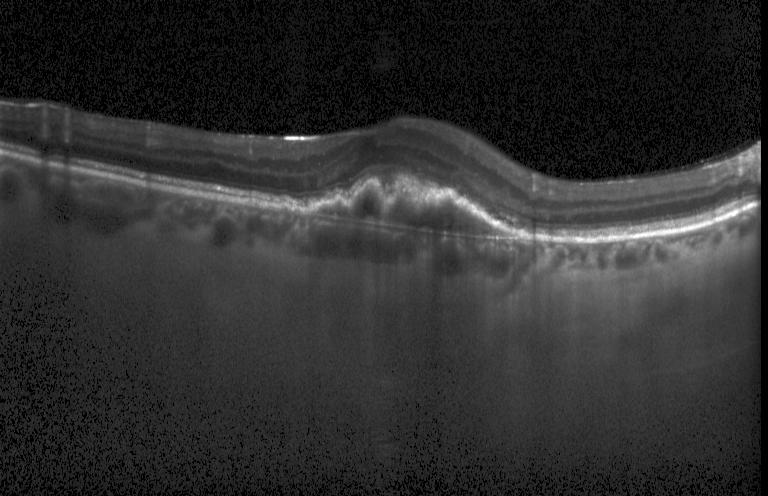
Heidelberg Spectralis OCT system; optical coherence tomography scan; through the macula. Diagnosis: a choroidal neovascular membrane.